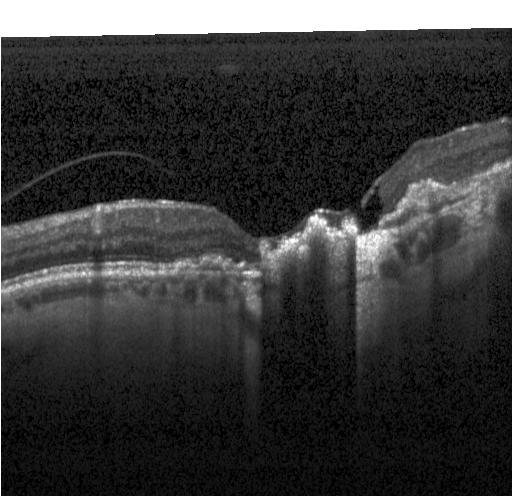

OCT line scan; fovea-centered — Assessment: a choroidal neovascular membrane.